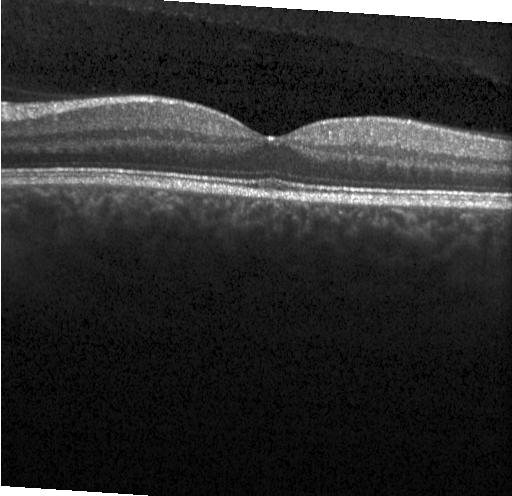
Macular OCT: no CNV, no DME, and no drusen.